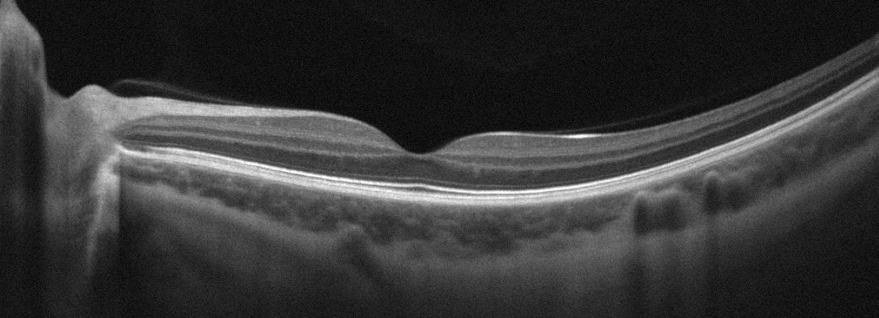
Finding: no AMD, DME, ERM, RAO, RVO, or VID.